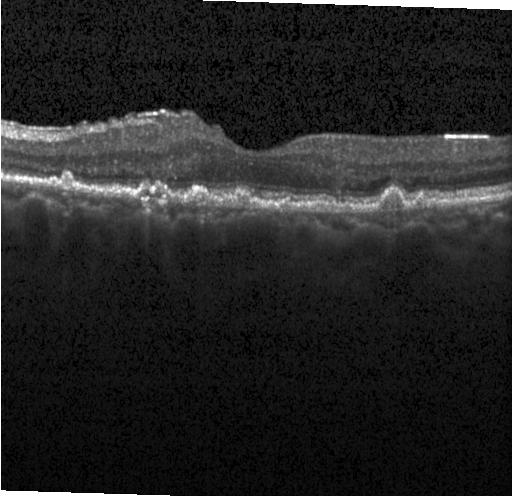 Spectral-domain optical coherence tomography, retinal OCT cross-section, horizontal scan through the fovea — Impression: multiple drusen.